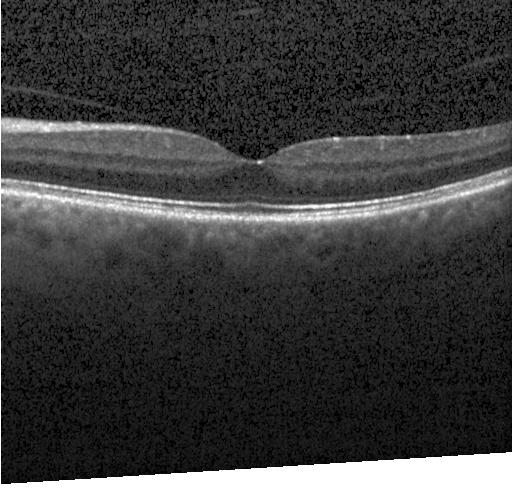

Heidelberg Spectralis OCT system · optical coherence tomography scan · through the macula · spectral-domain OCT. OCT finding: no evidence of CNV, DME, or drusen.